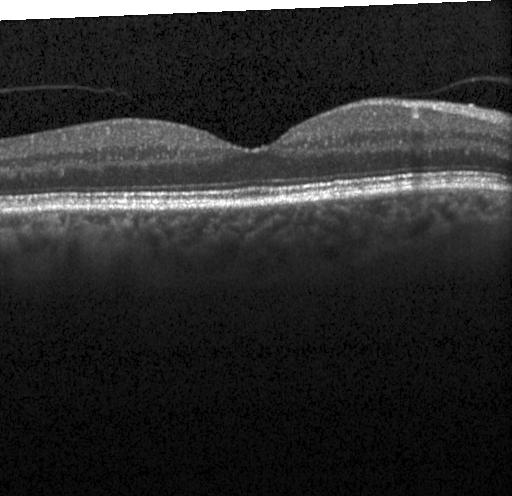 Retinal OCT B-scan.
Dx: no choroidal neovascularization, diabetic macular edema, or drusen.